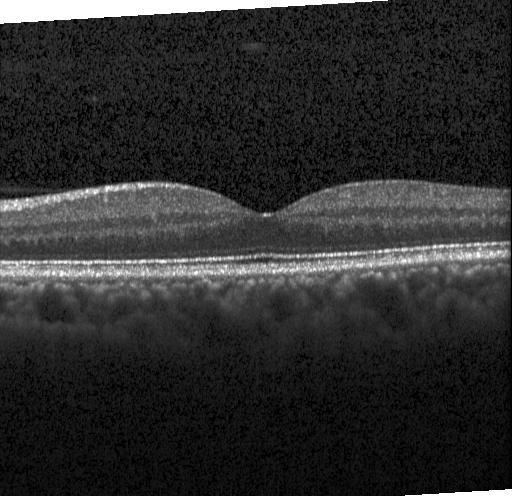
Optical coherence tomography scan.
Assessment: neither CNV, DME, nor drusen.